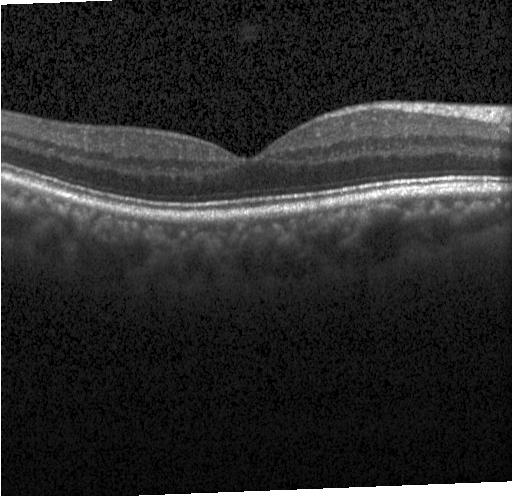

Acquired on a Heidelberg Spectralis; optical coherence tomography scan; SD-OCT. OCT finding: no evidence of choroidal neovascularization, diabetic macular edema, or drusen.